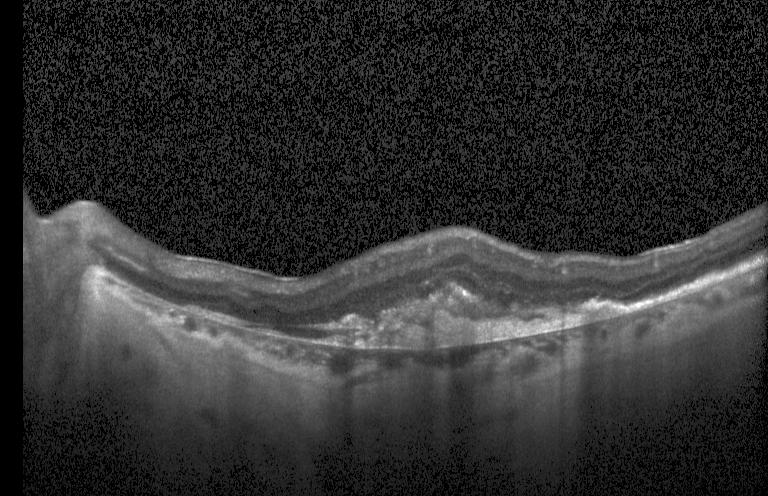

Spectral-domain OCT. Instrument: Heidelberg Spectralis. Optical coherence tomography scan
Impression: choroidal neovascularization.